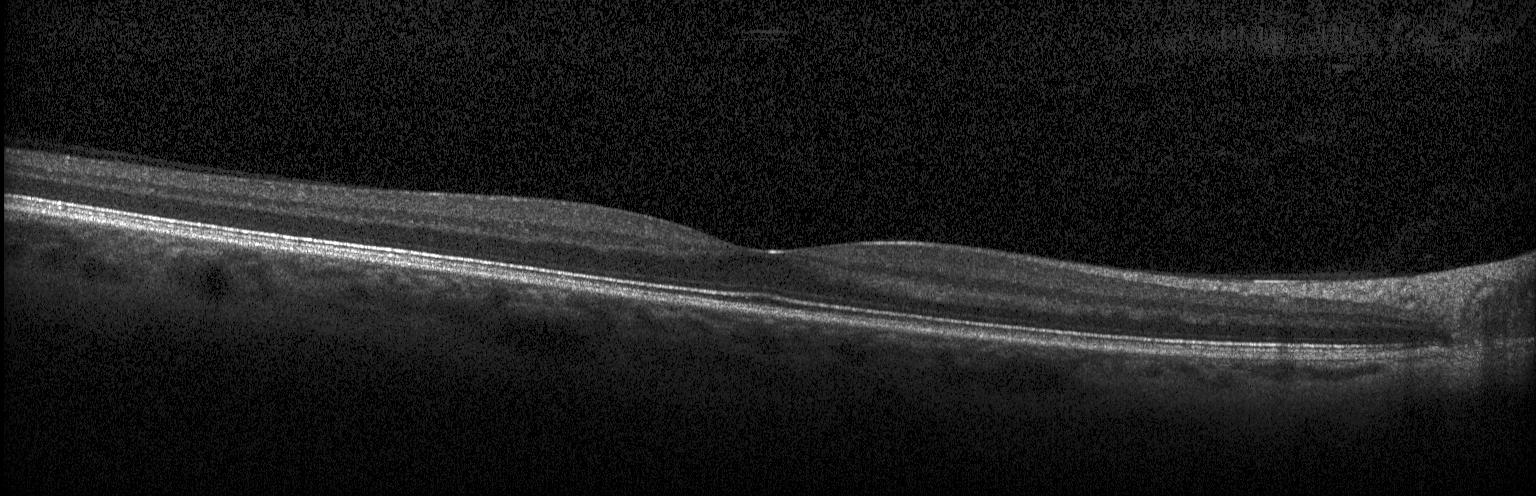

Assessment: no CNV, DME, or drusen.